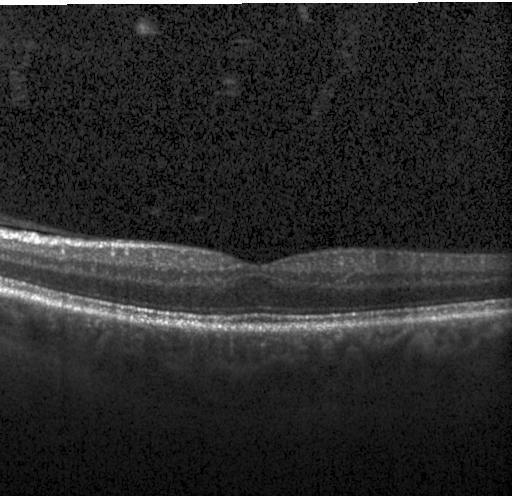 Optical coherence tomography B-scan
Finding: no evidence of choroidal neovascularization, diabetic macular edema, or drusen.